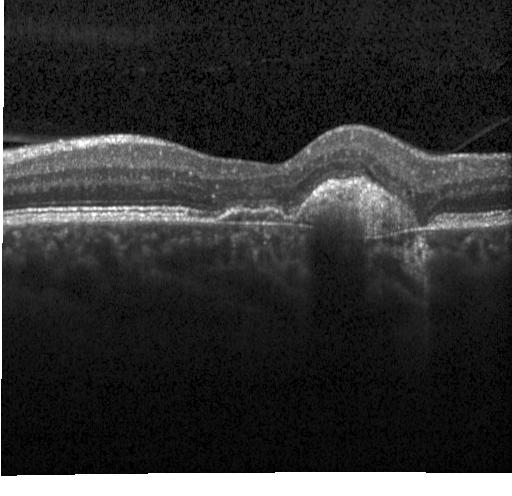
Retinal OCT cross-section showing a choroidal neovascular membrane.